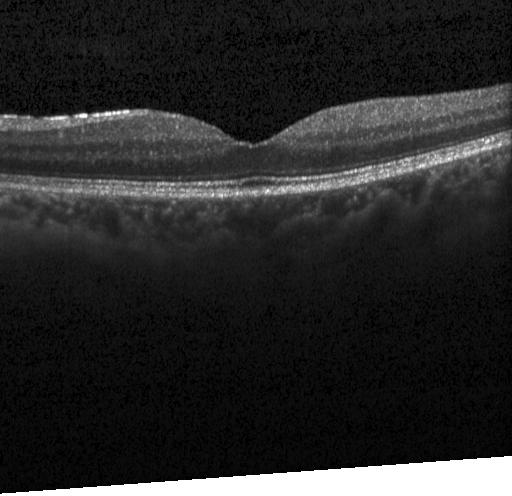
Retinal OCT B-scan · instrument: Heidelberg Spectralis — Dx: no evidence of choroidal neovascularization, diabetic macular edema, or drusen.